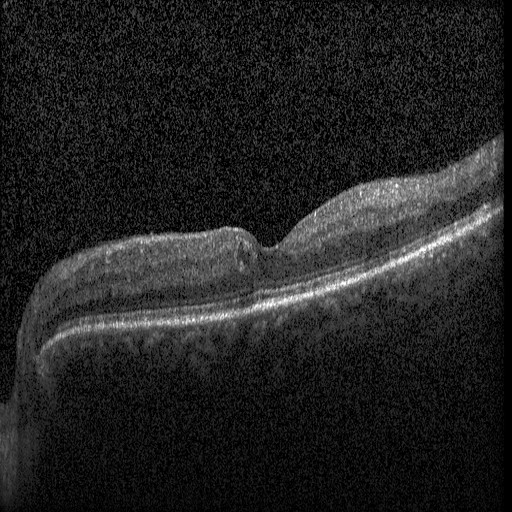
Impression: DME.